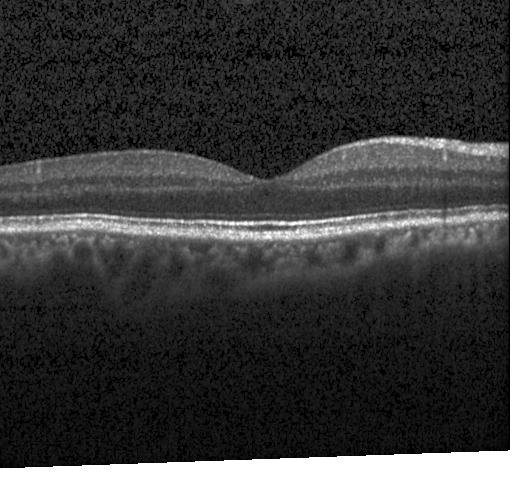

This B-scan demonstrates neither choroidal neovascularization, diabetic macular edema, nor drusen.